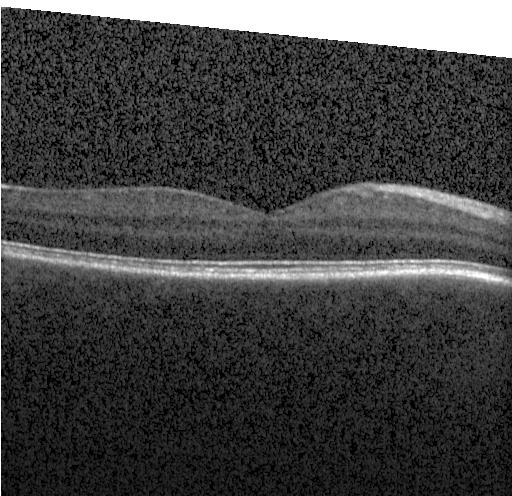 The scan shows no evidence of CNV, DME, or drusen.